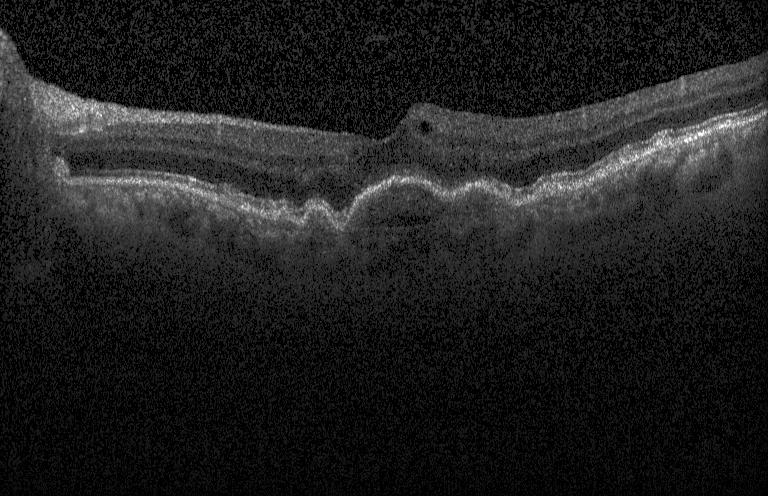
Macular OCT: a choroidal neovascular membrane.